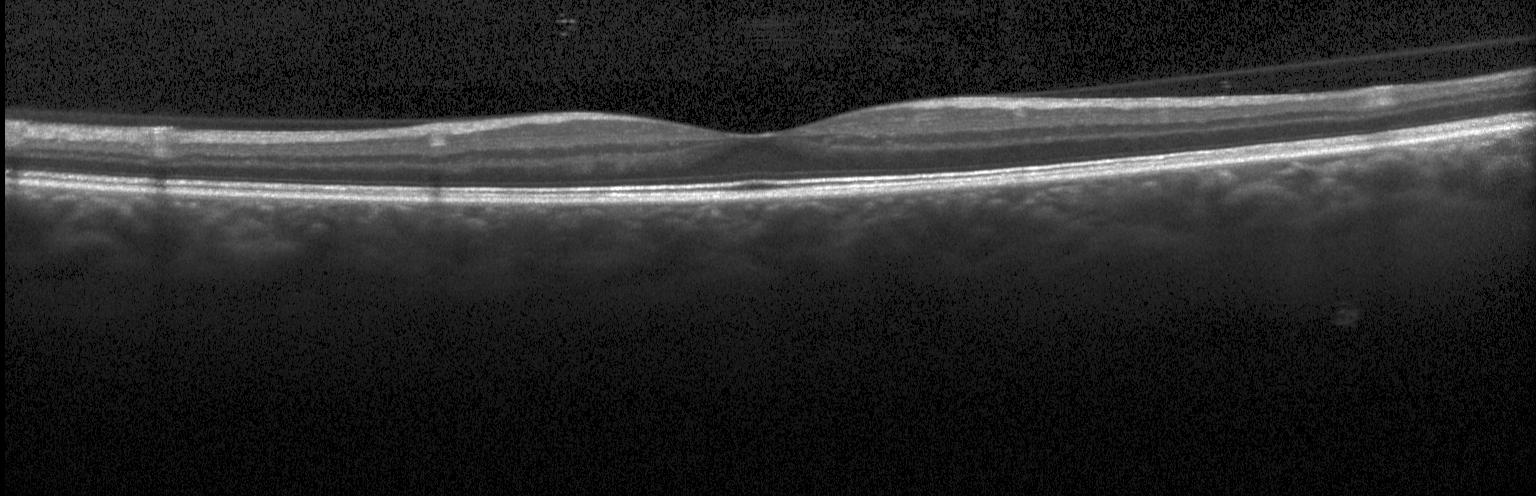
Dx: neither choroidal neovascularization, diabetic macular edema, nor drusen.